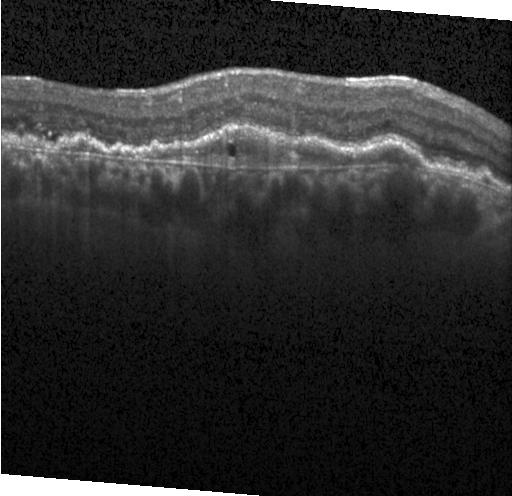

Retinal OCT cross-section; macular scan.
This B-scan demonstrates a choroidal neovascular membrane.